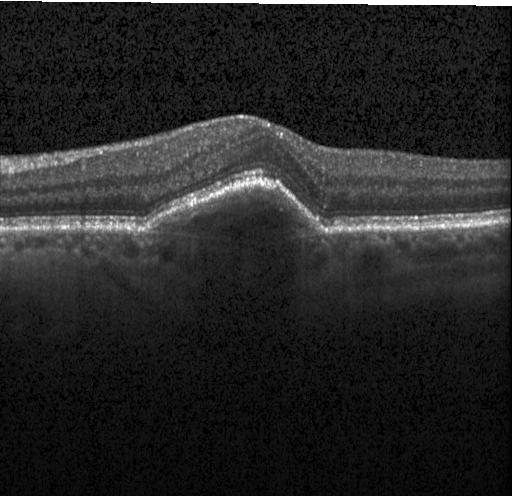

Optical coherence tomography scan · centered on the fovea · spectral-domain OCT.
OCT finding: a choroidal neovascular membrane.